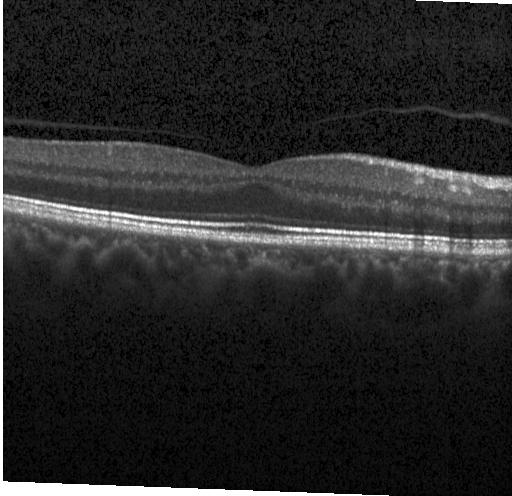
Optical coherence tomography scan. Diagnosis: neither choroidal neovascularization, diabetic macular edema, nor drusen.